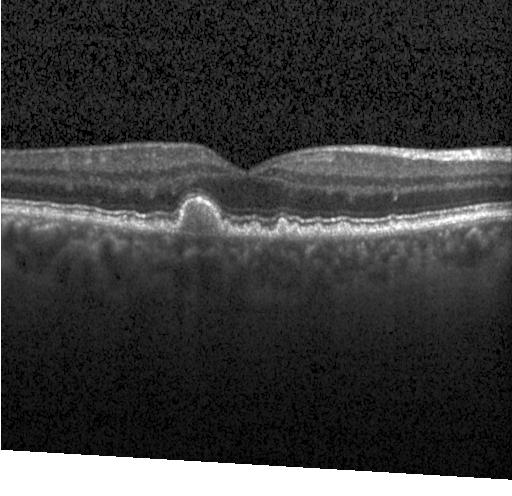 Fovea-centered, retinal OCT B-scan
A choroidal neovascular membrane.